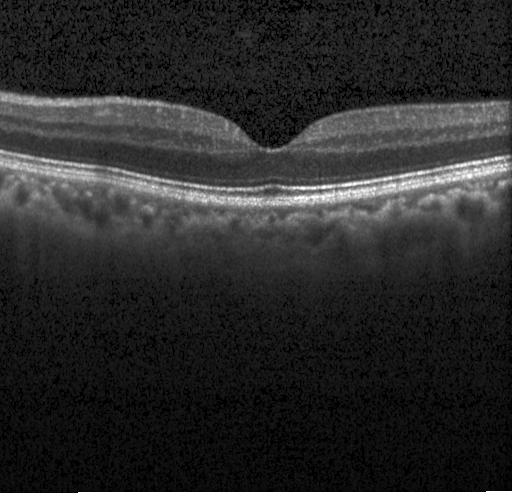
Spectral-domain OCT; retinal OCT B-scan; through the macula; acquired on a Heidelberg Spectralis — Diagnosis: no choroidal neovascularization, diabetic macular edema, or drusen.